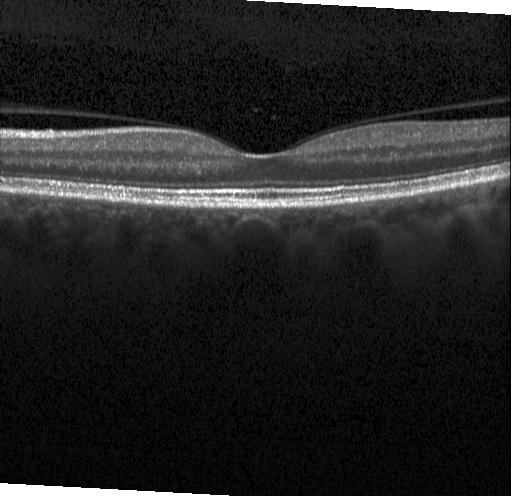
OCT B-scan. No CNV, no DME, and no drusen.